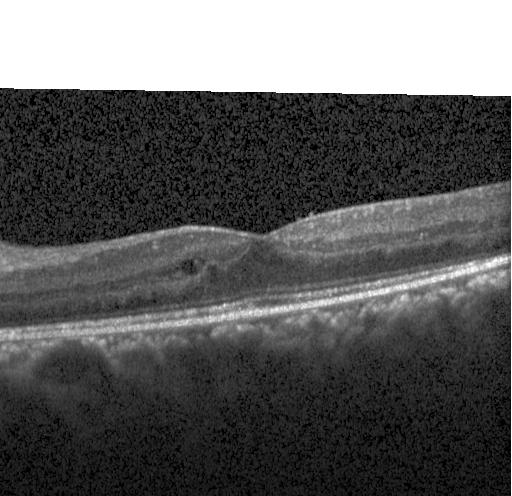

Through the macula; optical coherence tomography B-scan
DME.